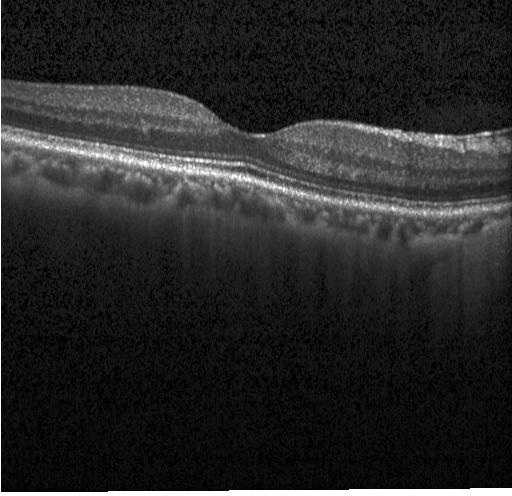 Acquired on a Heidelberg Spectralis. Centered on the fovea. Retinal OCT B-scan. OCT finding: no CNV, DME, or drusen.